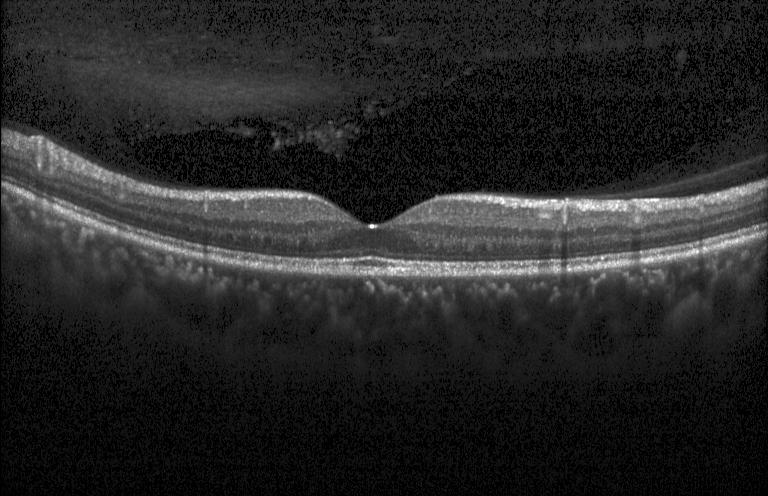 Heidelberg Spectralis OCT system. OCT line scan.
Impression: neither choroidal neovascularization, diabetic macular edema, nor drusen.